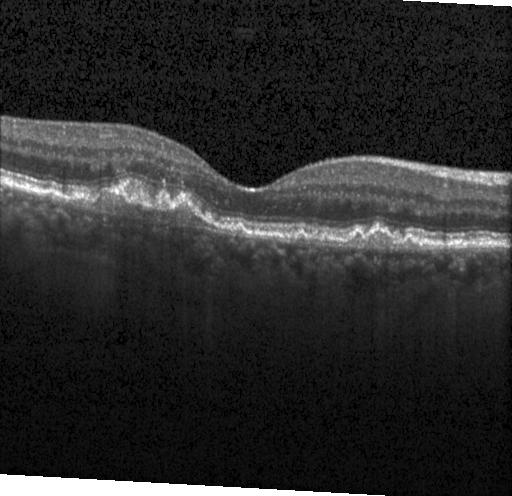
Choroidal neovascularization.